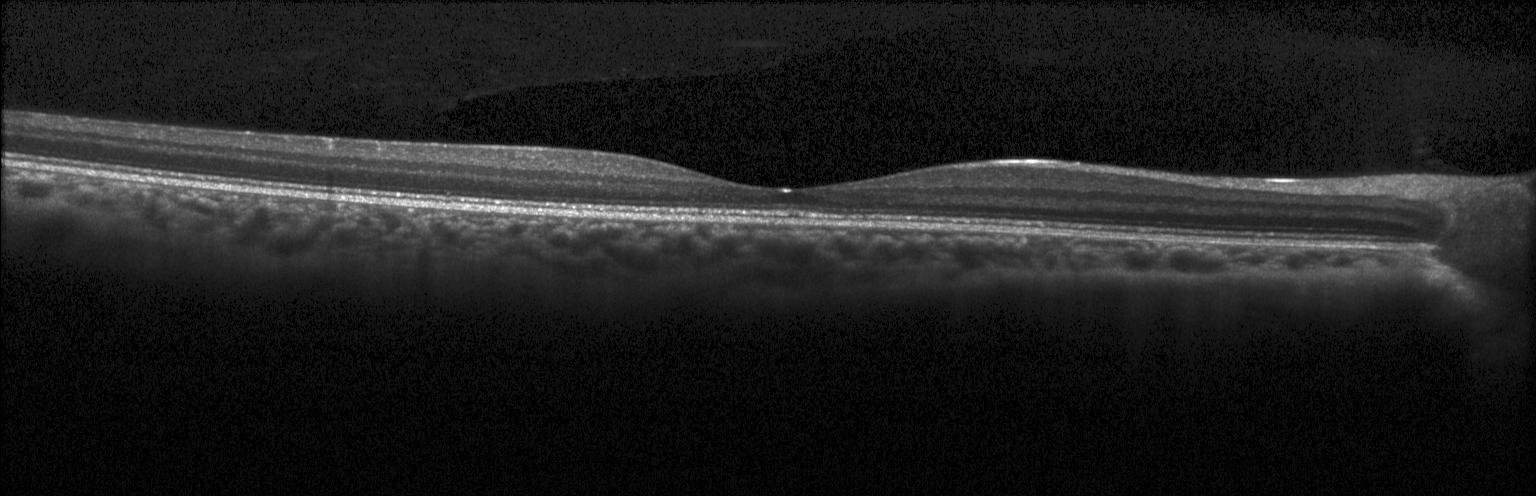 Macular OCT: no evidence of CNV, DME, or drusen.